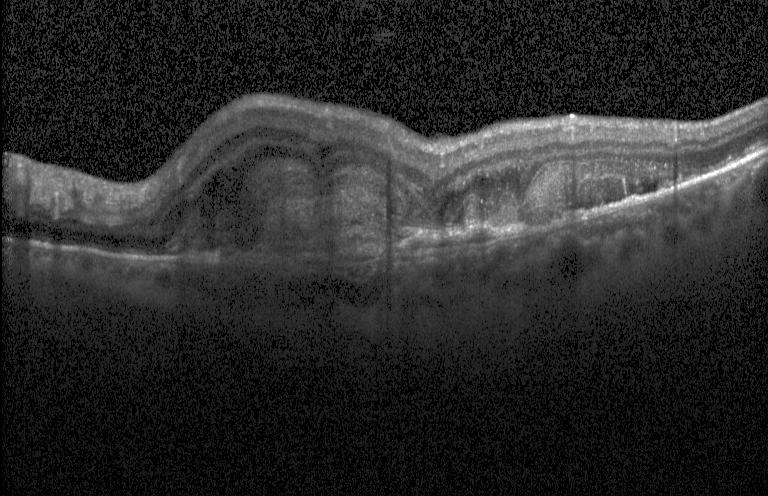 Impression: a choroidal neovascular membrane.